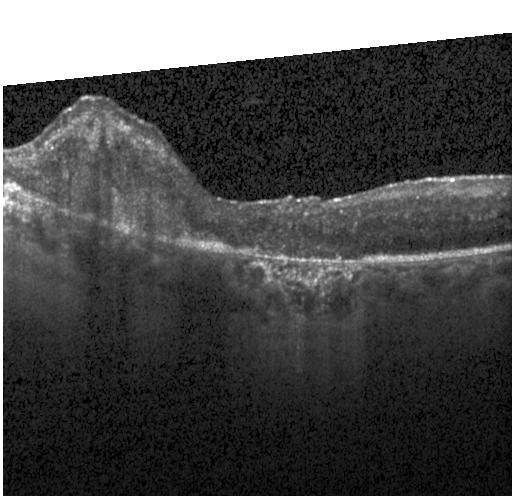
Assessment: CNV.